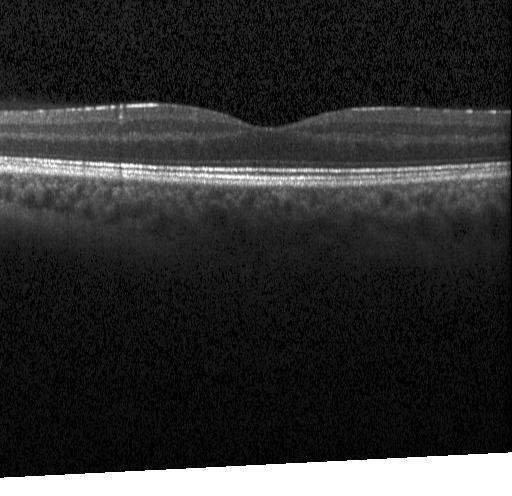

SD-OCT; OCT line scan; acquired on a Heidelberg Spectralis.
Finding: no choroidal neovascularization, diabetic macular edema, or drusen.